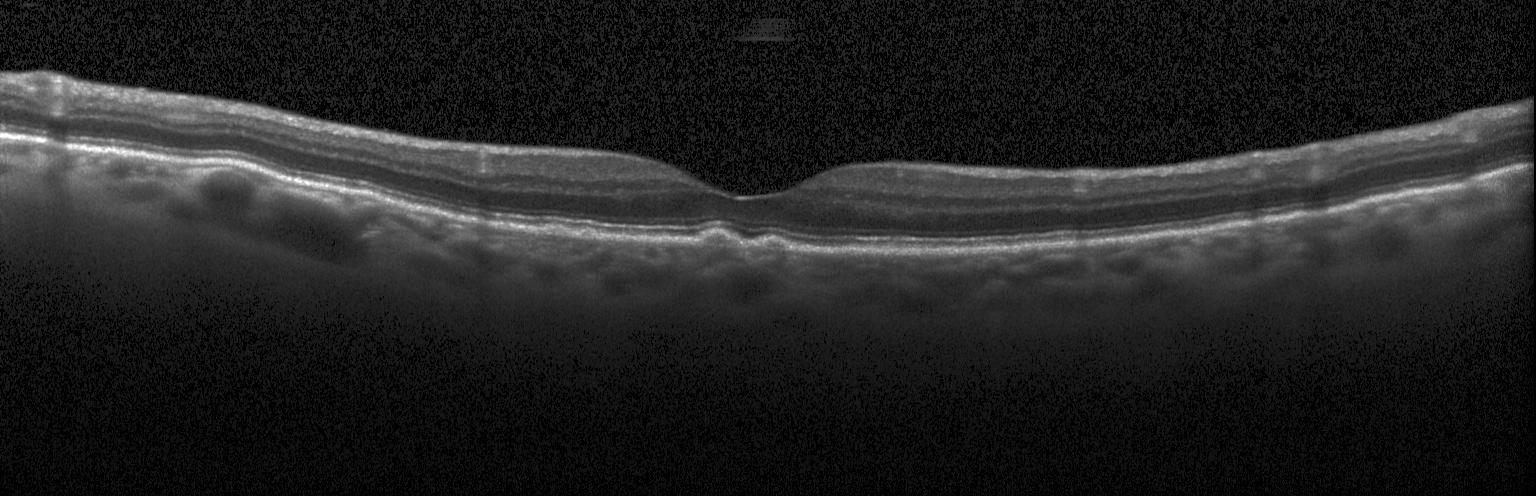

Optical coherence tomography B-scan — Impression: multiple drusen.